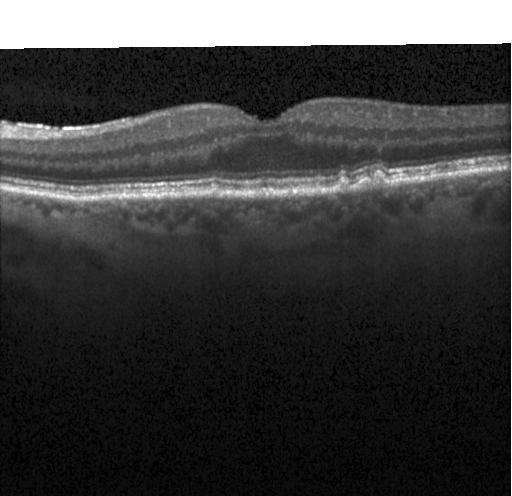

Dx: multiple drusen.